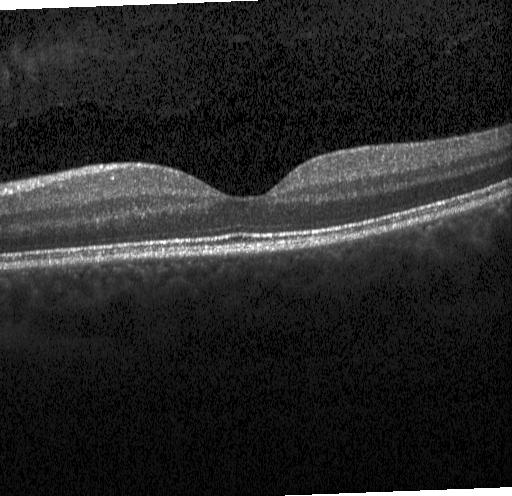

Diagnosis: no evidence of choroidal neovascularization, diabetic macular edema, or drusen.